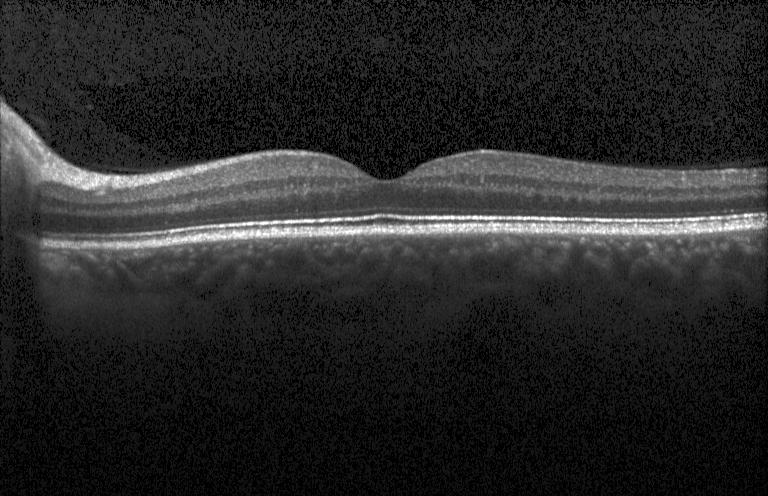

Diagnosis: no choroidal neovascularization, no diabetic macular edema, and no drusen.